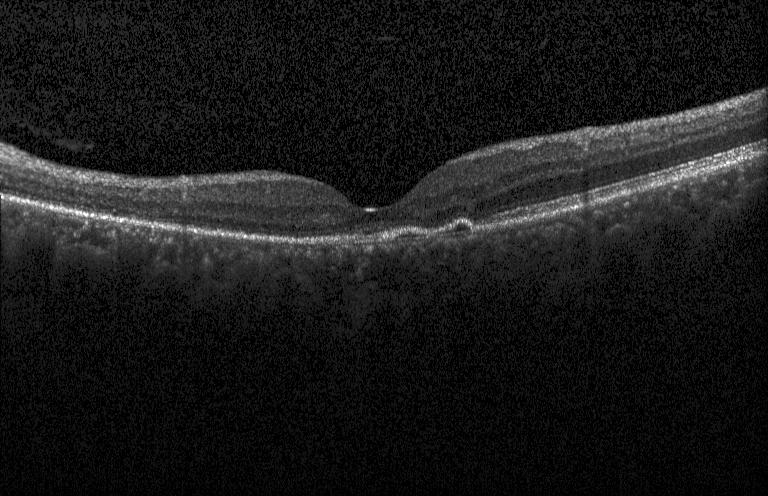
Dx: choroidal neovascularization (CNV).